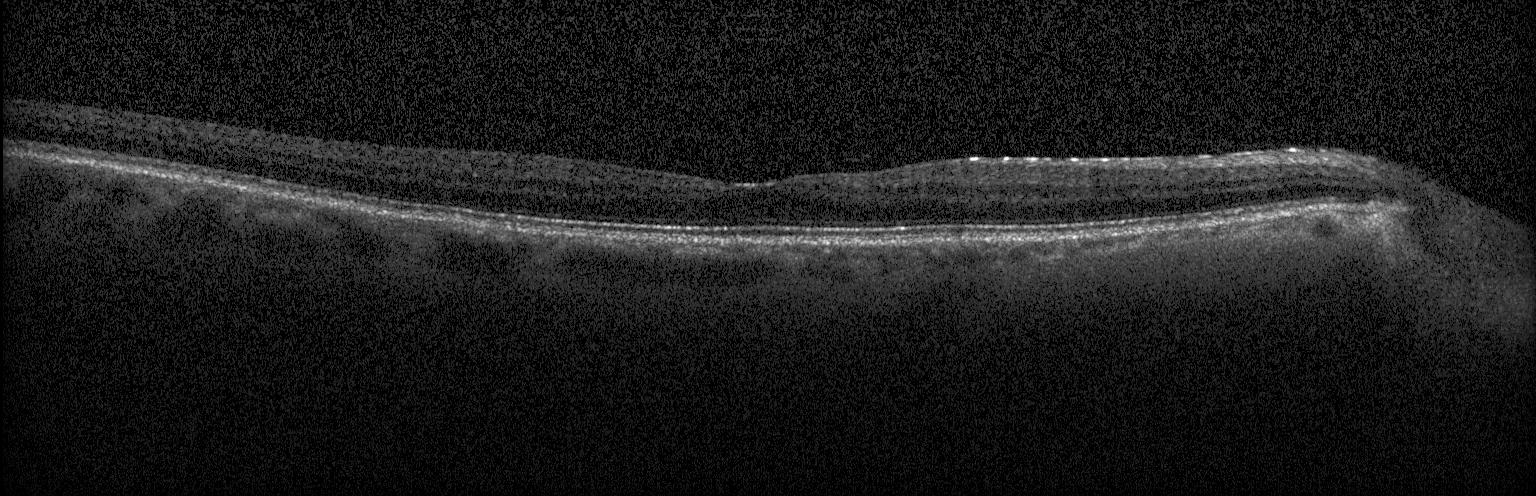
OCT scan showing no choroidal neovascularization, diabetic macular edema, or drusen.